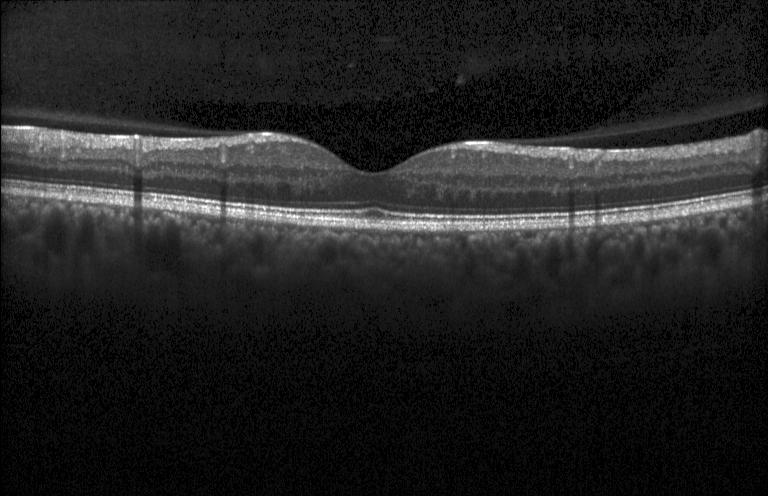 Finding: no CNV, no DME, and no drusen.